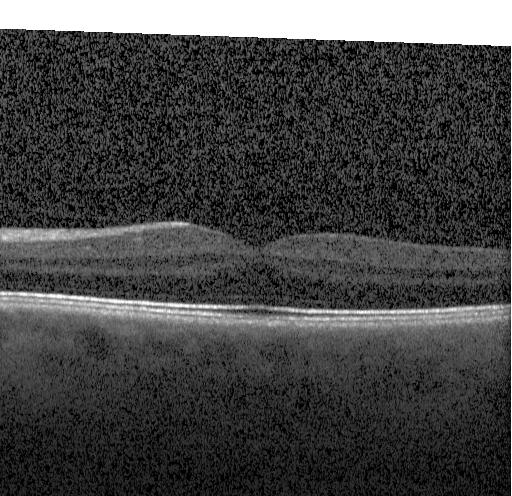

Heidelberg Spectralis OCT system · macular scan · retinal OCT cross-section. Macular OCT: no choroidal neovascularization, no diabetic macular edema, and no drusen.